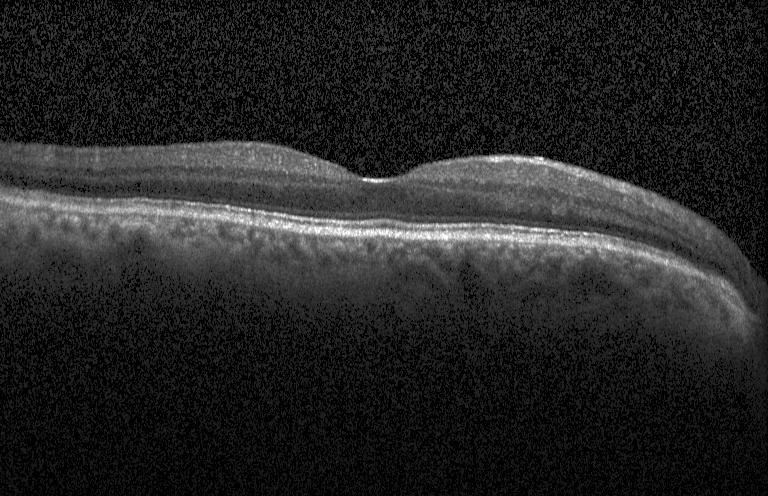
Fovea-centered; OCT B-scan; Heidelberg Spectralis OCT system — OCT finding: no choroidal neovascularization, diabetic macular edema, or drusen.